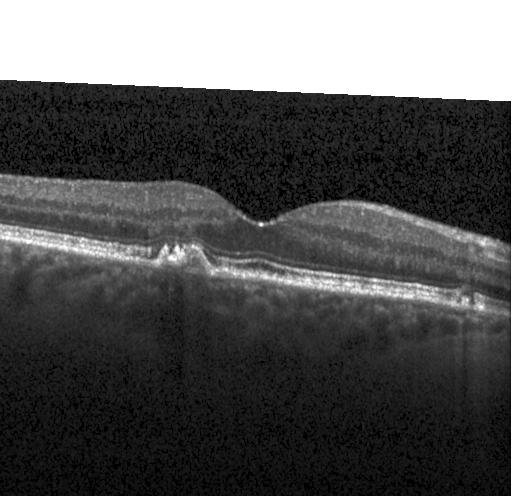 OCT finding: multiple drusen.